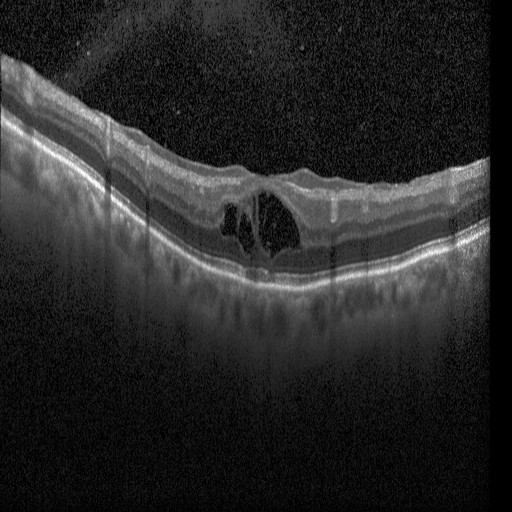
Optical coherence tomography scan
Macular OCT: DME.